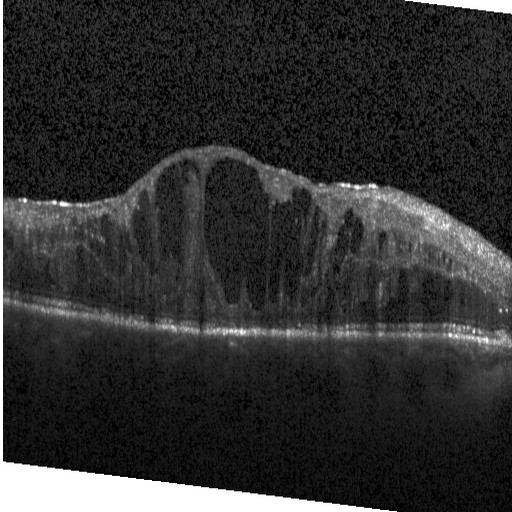
Heidelberg Spectralis OCT system; spectral-domain OCT; horizontal scan through the fovea; optical coherence tomography scan
Impression: diabetic macular edema.